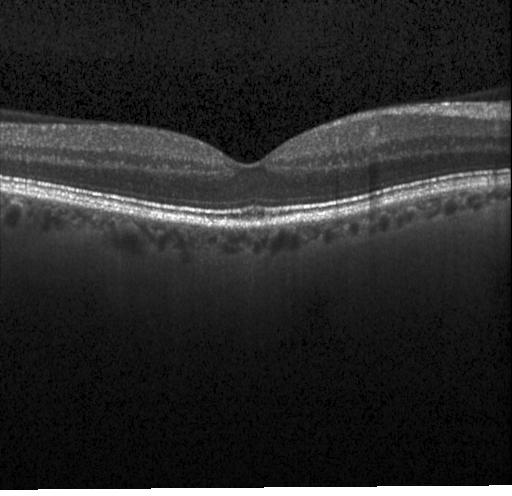 Through the macula; OCT B-scan. Diagnosis: no CNV, DME, or drusen.